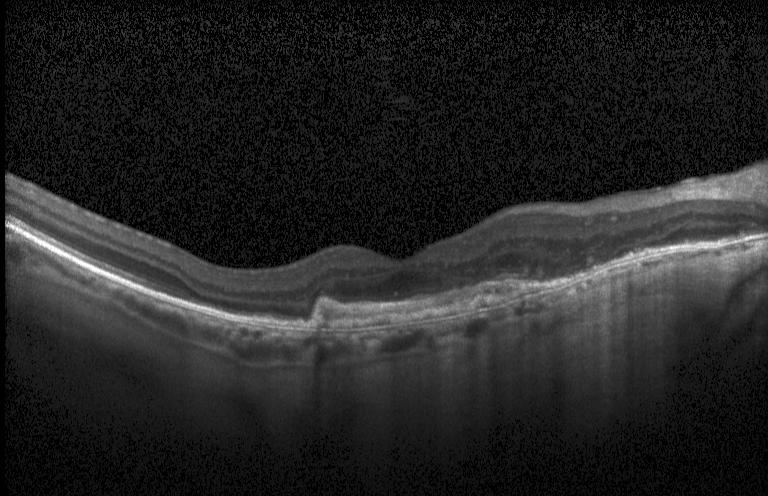 The scan shows a choroidal neovascular membrane.